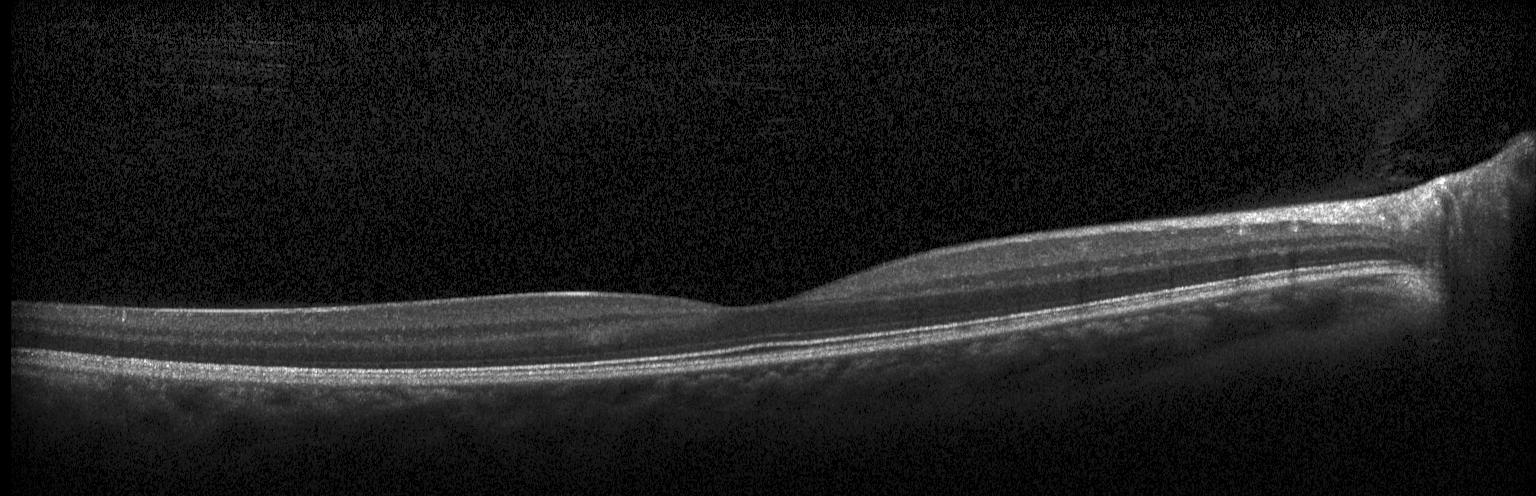
Spectral-domain optical coherence tomography. Fovea-centered. Retinal OCT cross-section. Heidelberg Spectralis OCT system. No choroidal neovascularization, diabetic macular edema, or drusen.